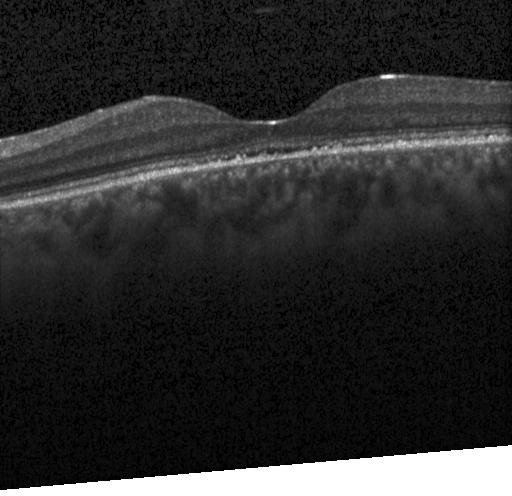

Diagnosis: no choroidal neovascularization, no diabetic macular edema, and no drusen.